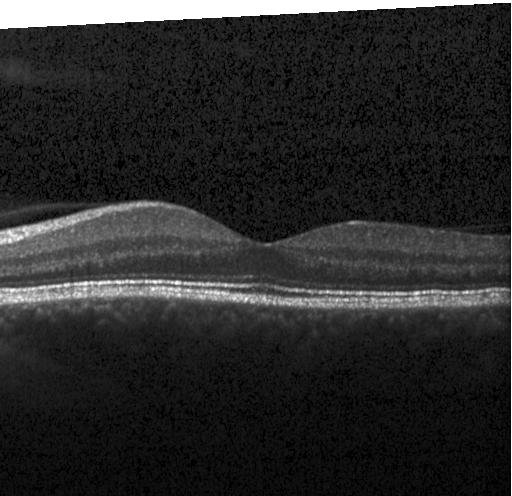

Spectral-domain optical coherence tomography, instrument: Heidelberg Spectralis, OCT line scan, through the macula.
The scan shows no choroidal neovascularization, no diabetic macular edema, and no drusen.